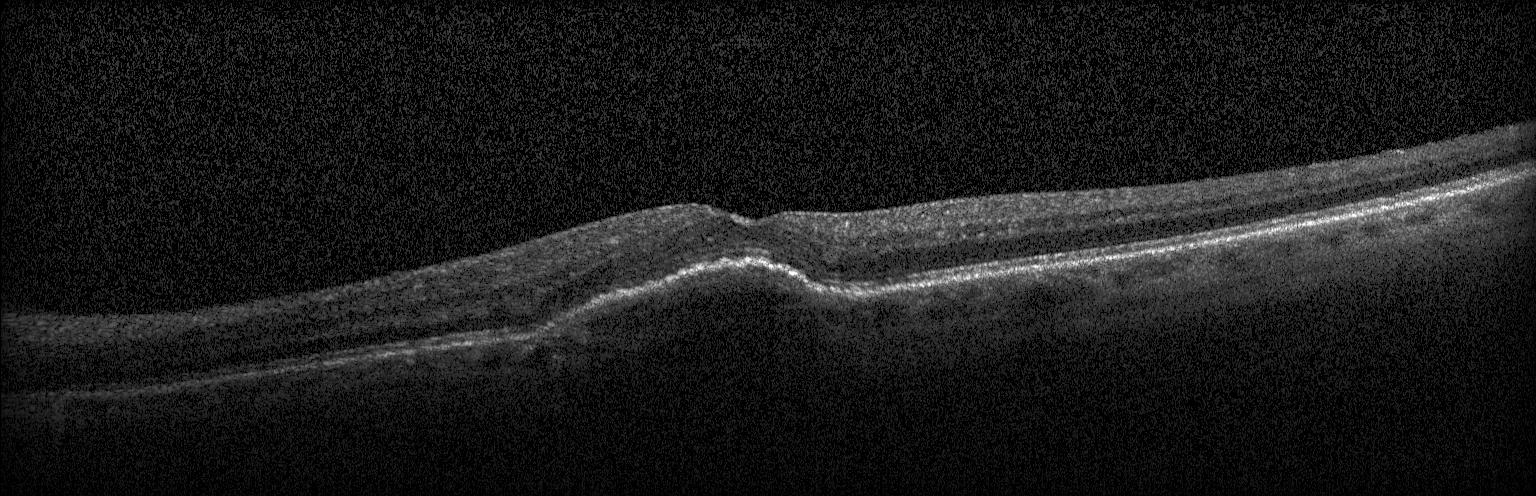
Optical coherence tomography B-scan; centered on the fovea.
A choroidal neovascular membrane.